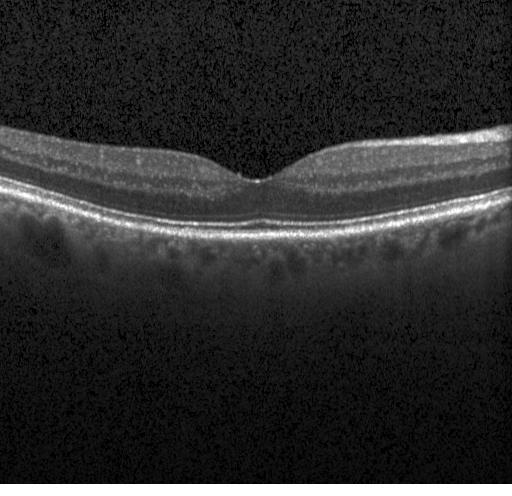 Finding: no CNV, DME, or drusen.